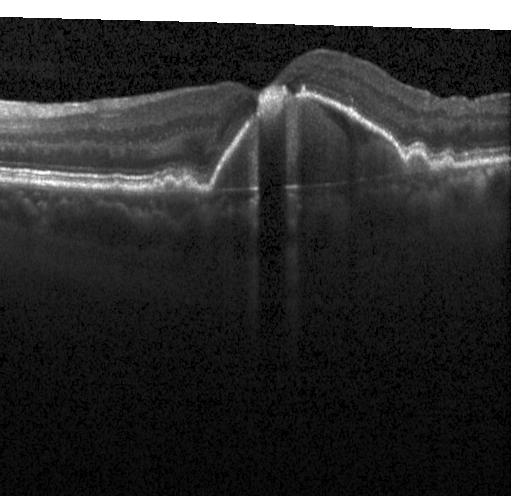
This B-scan demonstrates a choroidal neovascular membrane.